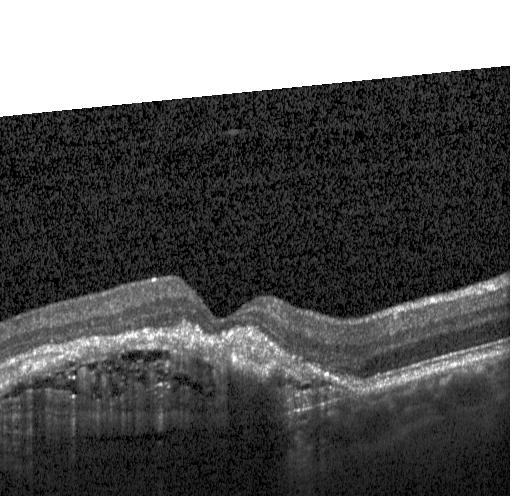
Heidelberg Spectralis; OCT line scan
Diagnosis: a choroidal neovascular membrane.